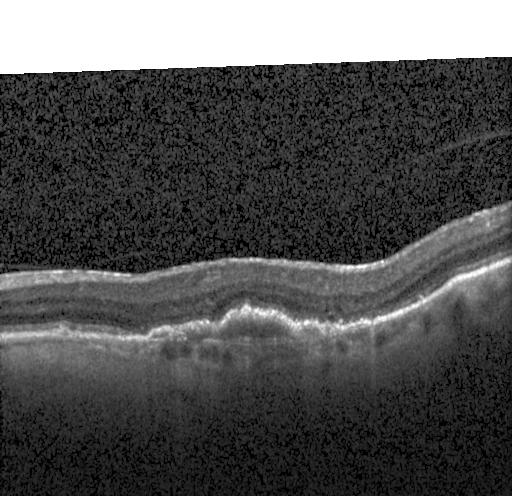
Horizontal scan through the fovea; Heidelberg Spectralis OCT system; OCT line scan. Finding: a choroidal neovascular membrane.